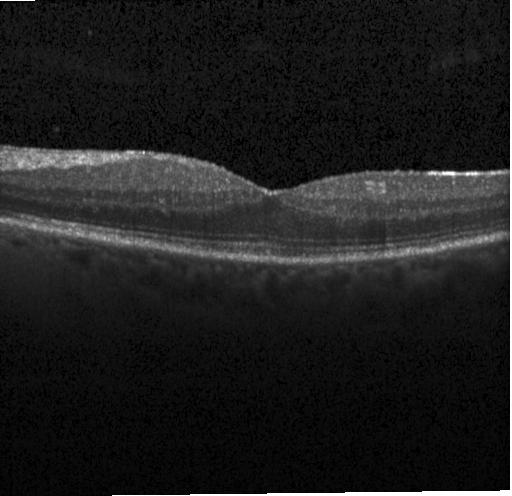 Spectral-domain optical coherence tomography, centered on the fovea, instrument: Heidelberg Spectralis, retinal OCT B-scan
Macular OCT: no choroidal neovascularization, diabetic macular edema, or drusen.